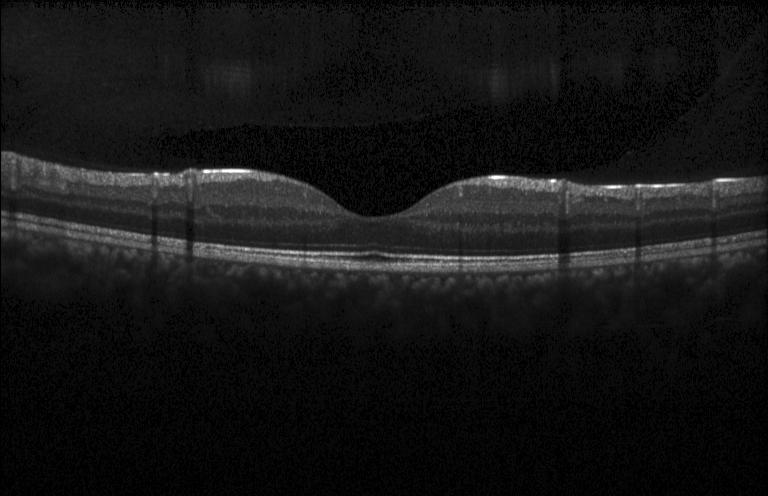

Retinal OCT cross-section · Heidelberg Spectralis
Dx: neither CNV, DME, nor drusen.